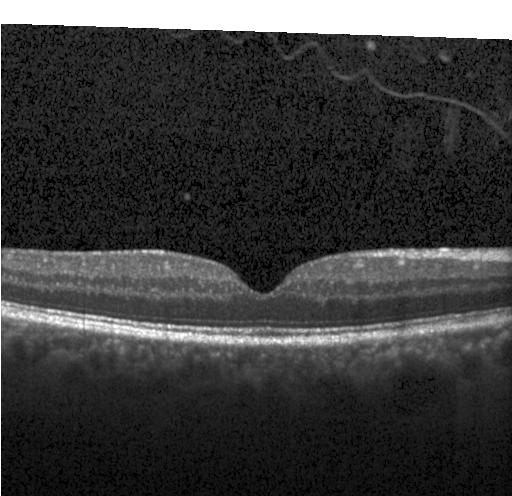

OCT B-scan · Heidelberg Spectralis · through the macula.
Assessment: no CNV, DME, or drusen.